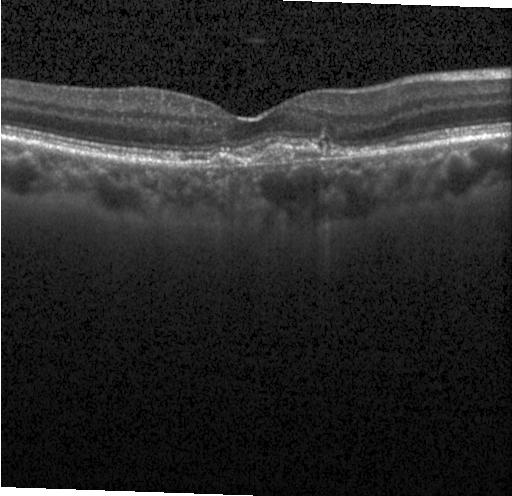

OCT B-scan showing choroidal neovascularization (CNV).